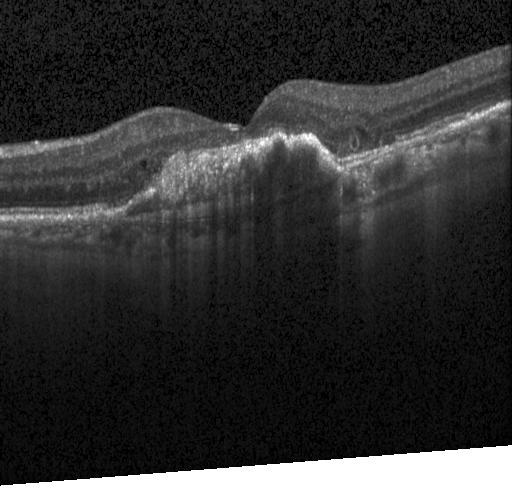 Instrument: Heidelberg Spectralis; through the macula; optical coherence tomography scan; spectral-domain optical coherence tomography.
Impression: a choroidal neovascular membrane.